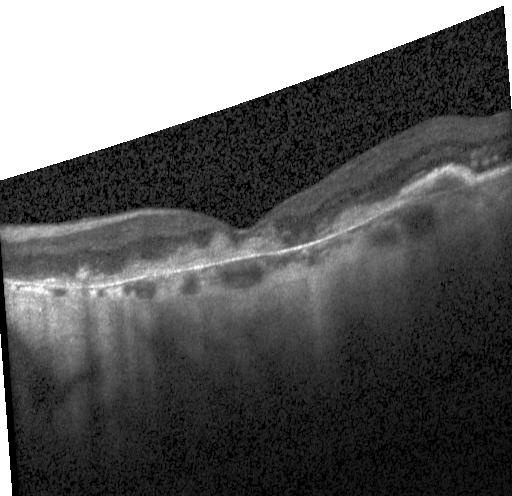
Finding: a choroidal neovascular membrane.